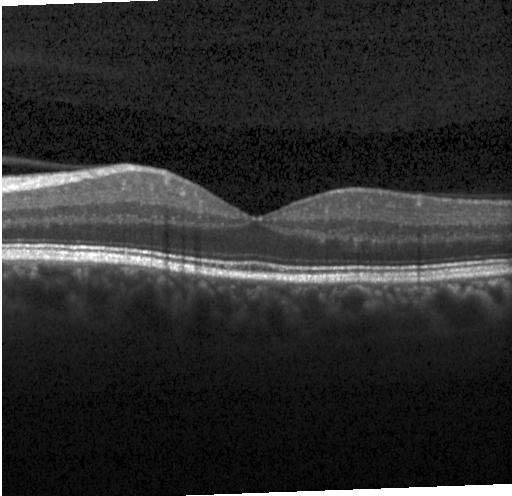 Heidelberg Spectralis OCT system, optical coherence tomography scan, fovea-centered
Diagnosis: no choroidal neovascularization, diabetic macular edema, or drusen.